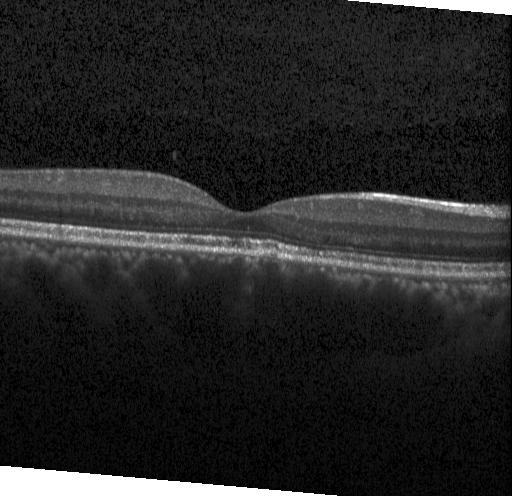
Spectral-domain optical coherence tomography · retinal OCT cross-section · Heidelberg Spectralis · horizontal scan through the fovea
Assessment: no choroidal neovascularization, no diabetic macular edema, and no drusen.